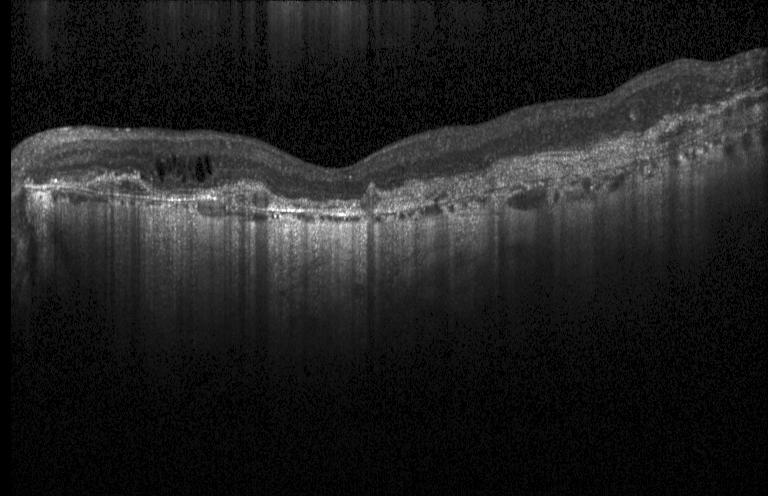

Spectral-domain OCT · OCT B-scan · macular scan. Finding: choroidal neovascularization.